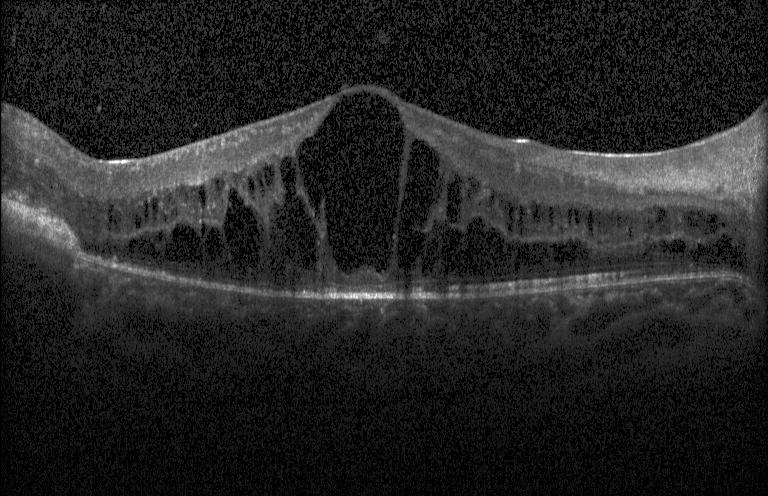

OCT finding: diabetic macular edema.